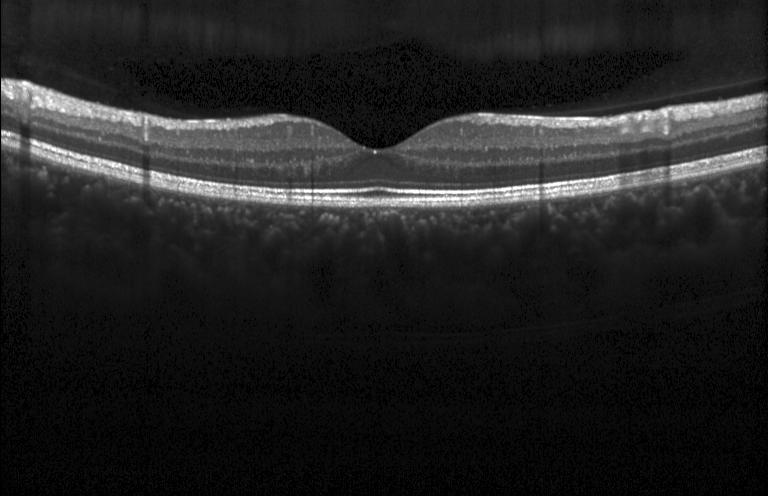 Heidelberg Spectralis; spectral-domain optical coherence tomography; through the macula; optical coherence tomography scan.
Diagnosis: no evidence of choroidal neovascularization, diabetic macular edema, or drusen.